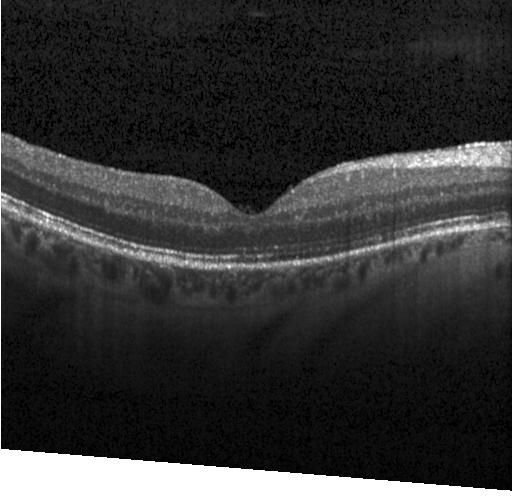

Spectral-domain optical coherence tomography, retinal OCT B-scan, instrument: Heidelberg Spectralis.
Diagnosis: no CNV, no DME, and no drusen.